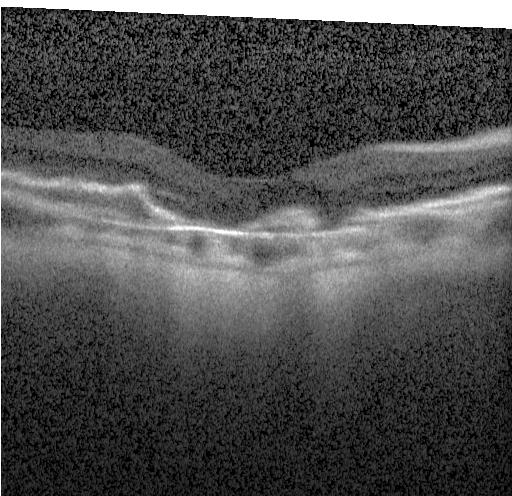
Macular OCT: CNV.